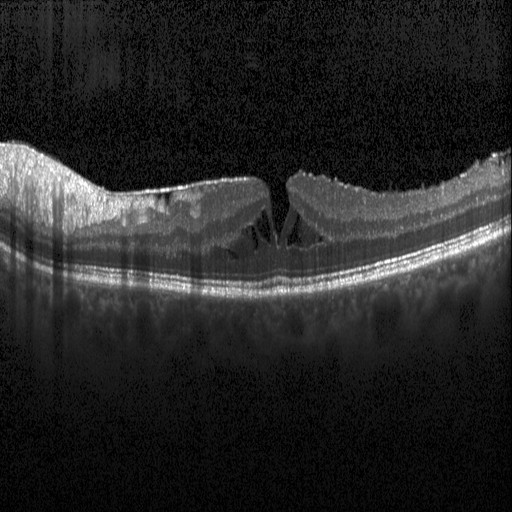 Dx: diabetic macular edema (DME).